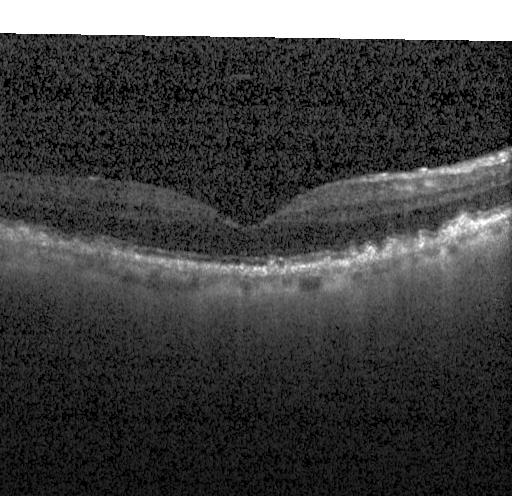

Retinal OCT cross-section. Heidelberg Spectralis. Impression: multiple drusen.